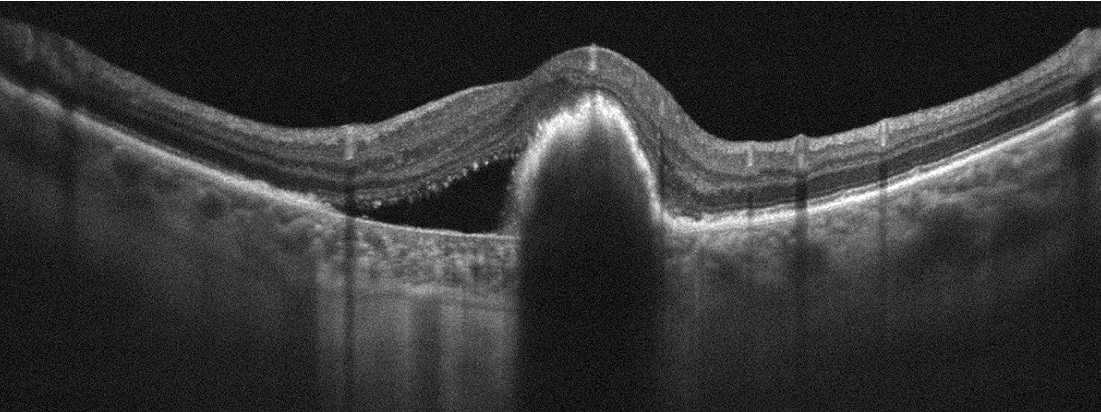

Macular OCT: AMD.